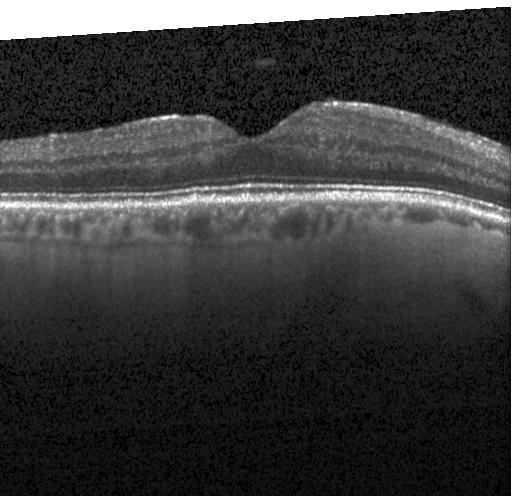
Diagnosis: no choroidal neovascularization, diabetic macular edema, or drusen.